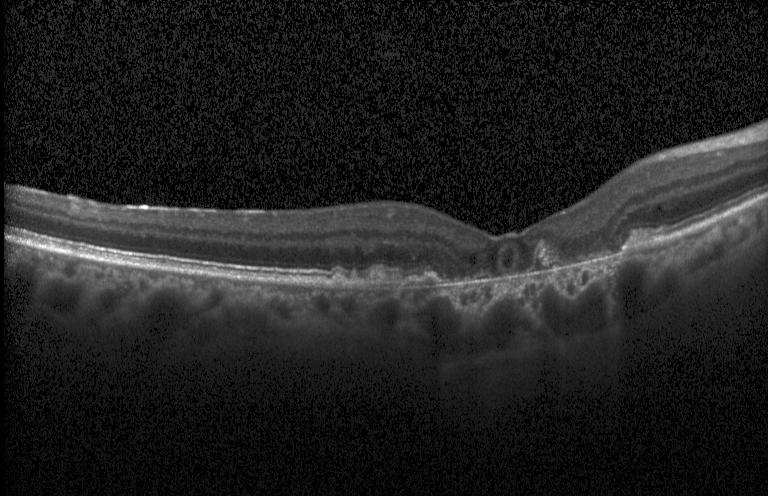

Optical coherence tomography scan. Heidelberg Spectralis OCT system. Spectral-domain optical coherence tomography — Diagnosis: a choroidal neovascular membrane.